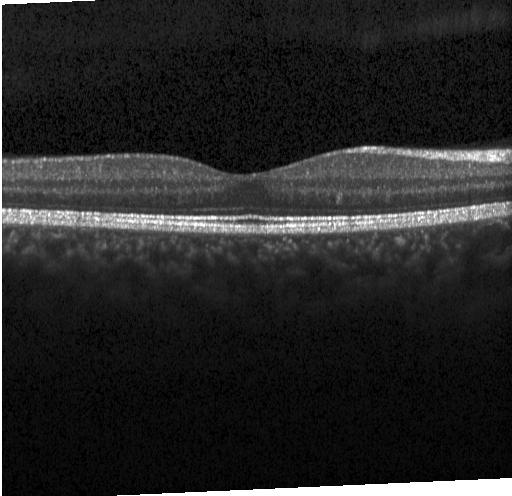 OCT finding: no evidence of CNV, DME, or drusen.